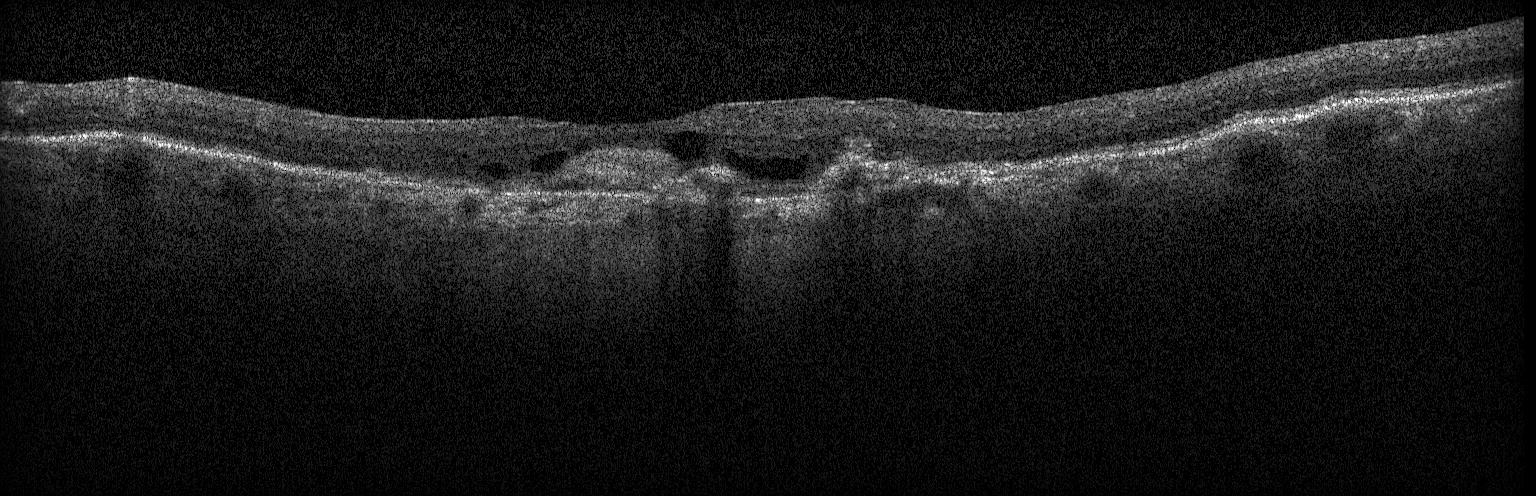

Impression: choroidal neovascularization.